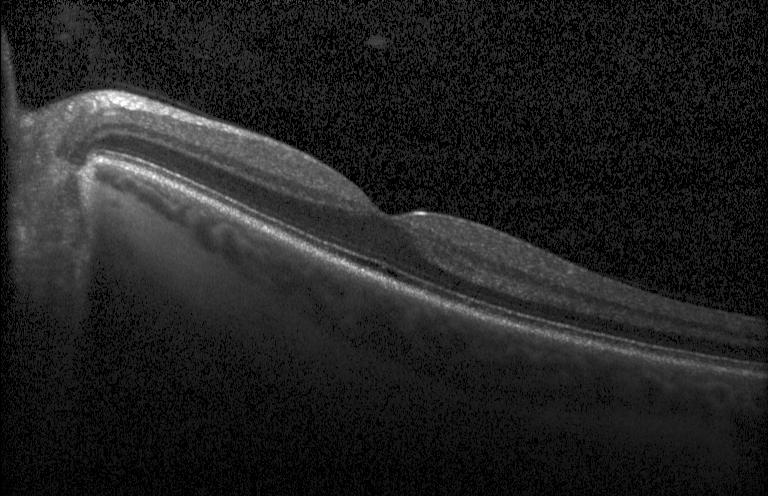

OCT B-scan showing no CNV, no DME, and no drusen.